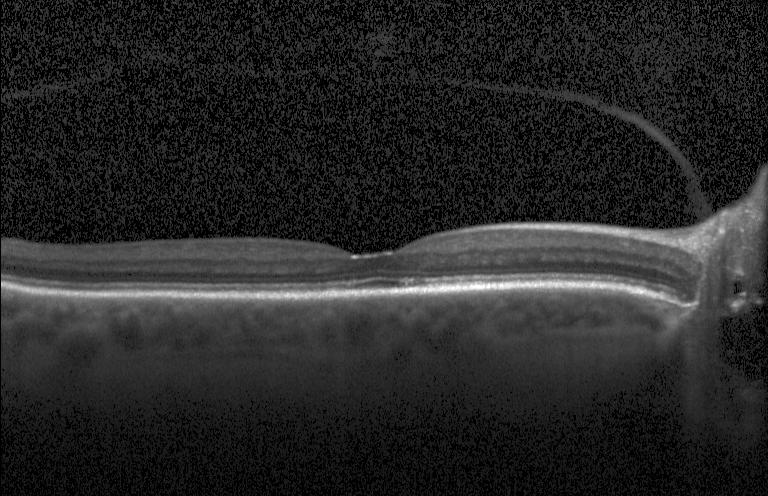 Heidelberg Spectralis OCT system, OCT B-scan, SD-OCT. The scan shows neither choroidal neovascularization, diabetic macular edema, nor drusen.